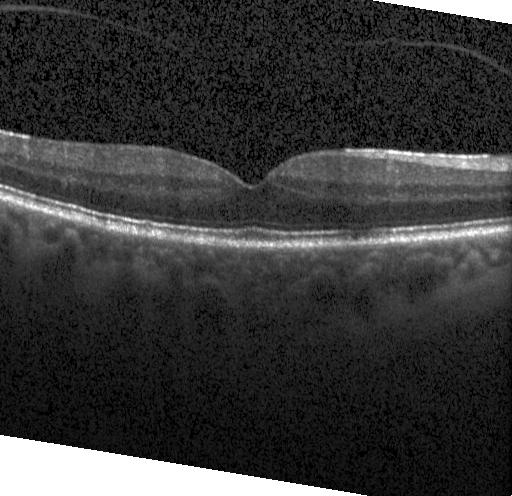 OCT line scan. Spectral-domain OCT. Heidelberg Spectralis OCT system
Diagnosis: no evidence of choroidal neovascularization, diabetic macular edema, or drusen.